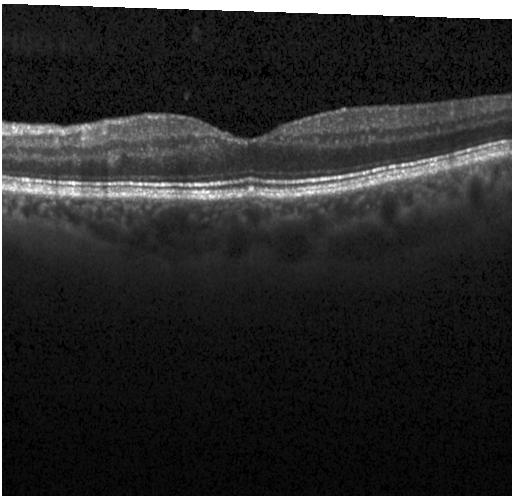
Spectral-domain optical coherence tomography · optical coherence tomography scan
Impression: neither choroidal neovascularization, diabetic macular edema, nor drusen.